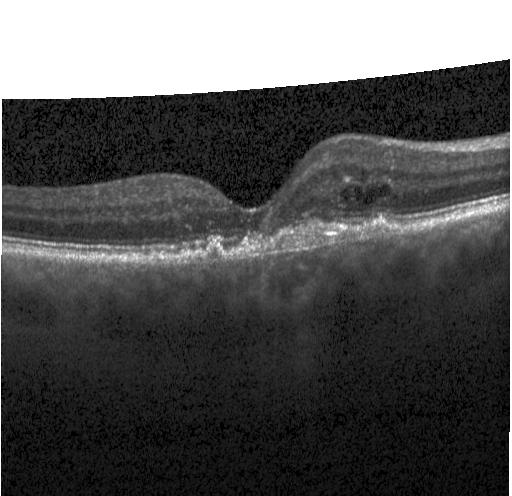

Diagnosis: a choroidal neovascular membrane.